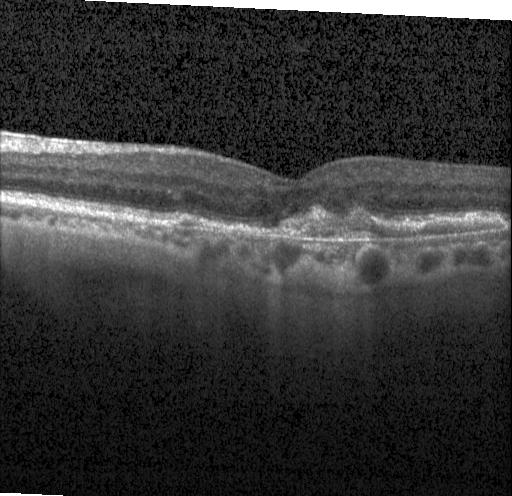 Macular OCT demonstrating a choroidal neovascular membrane.